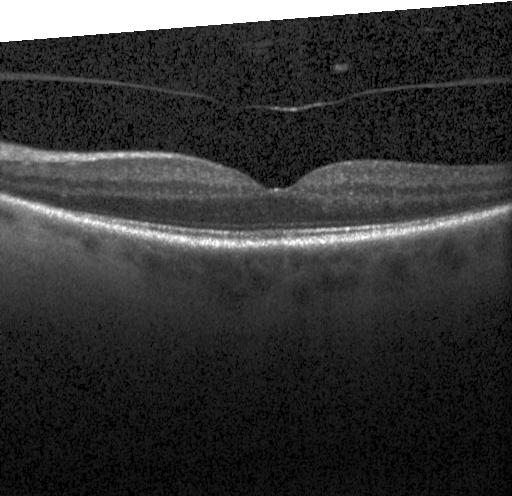

Spectral-domain optical coherence tomography, retinal OCT B-scan, acquired on a Heidelberg Spectralis. Diagnosis: no CNV, DME, or drusen.